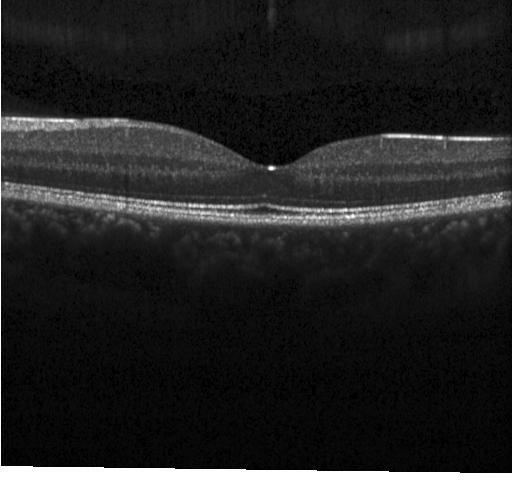
OCT scan showing neither choroidal neovascularization, diabetic macular edema, nor drusen.